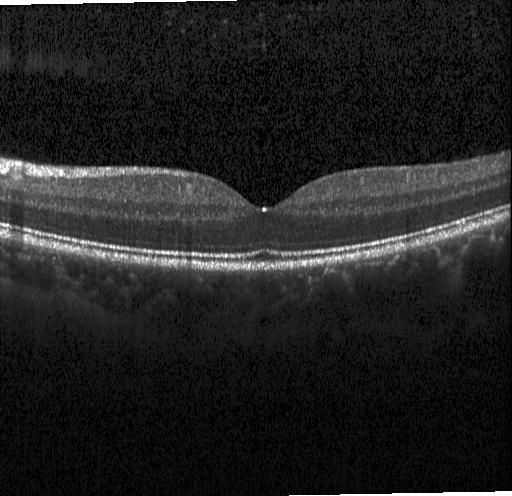 Spectral-domain optical coherence tomography. Heidelberg Spectralis OCT system. Centered on the fovea. Retinal OCT cross-section.
Diagnosis: neither choroidal neovascularization, diabetic macular edema, nor drusen.